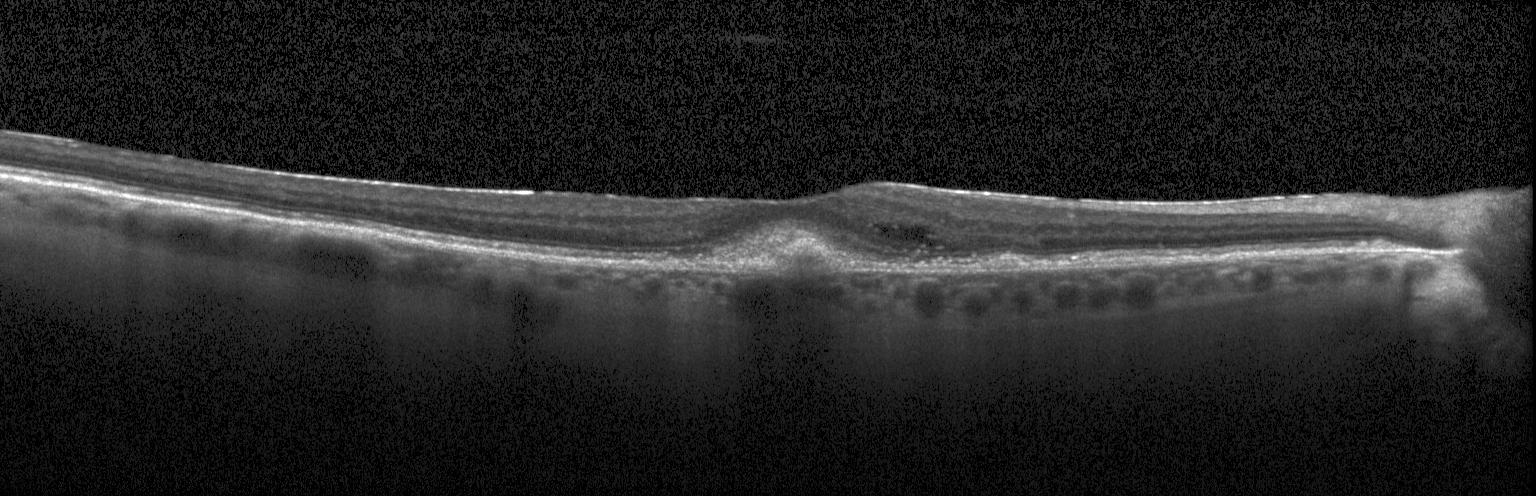

Optical coherence tomography scan. Macular OCT: choroidal neovascularization.